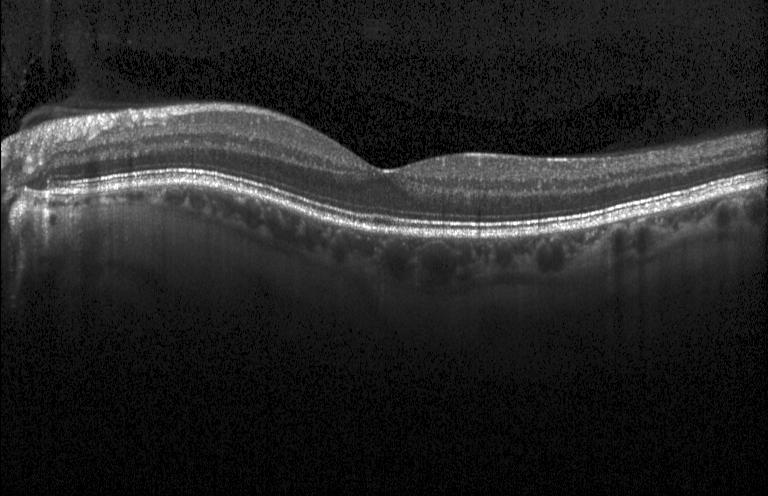

Macular scan. SD-OCT. Heidelberg Spectralis OCT system. Optical coherence tomography B-scan.
No evidence of choroidal neovascularization, diabetic macular edema, or drusen.